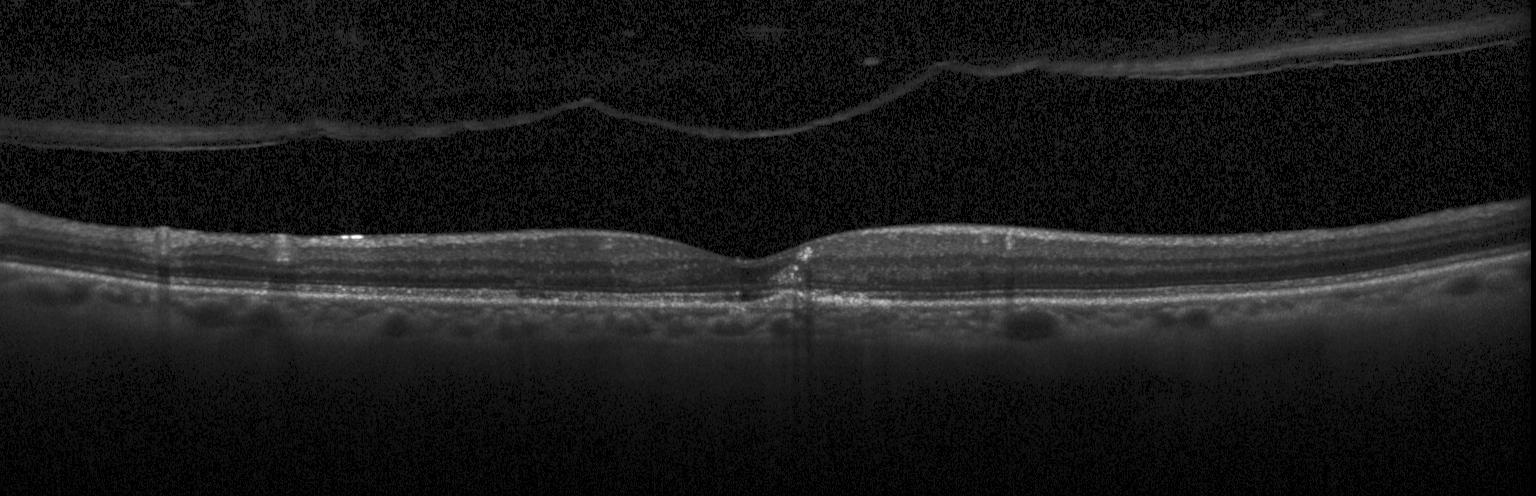

Impression: a choroidal neovascular membrane.